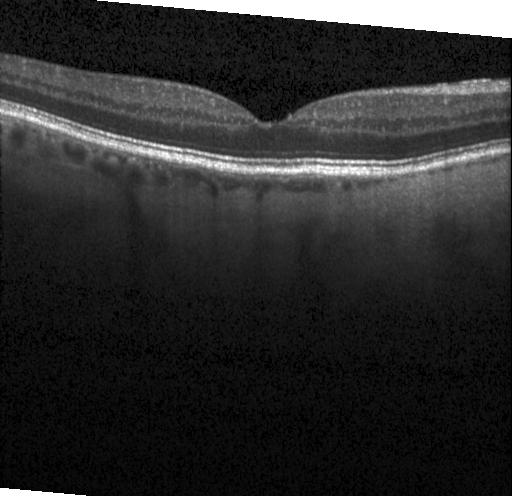

Finding: no CNV, no DME, and no drusen.